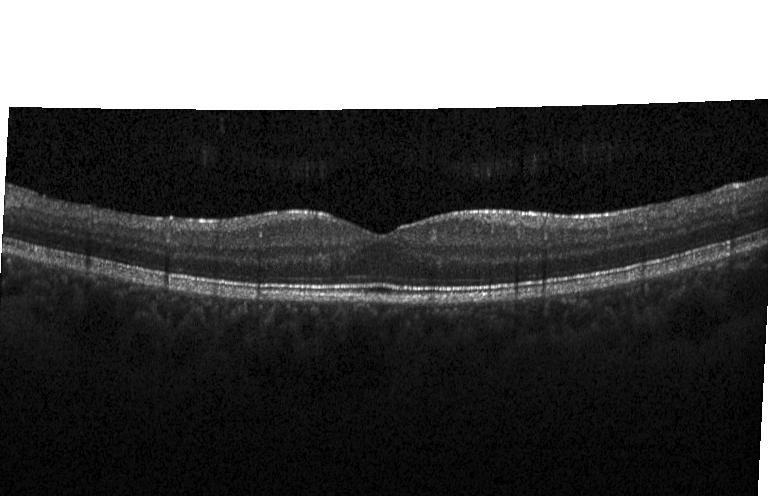

Instrument: Heidelberg Spectralis; through the macula; SD-OCT; OCT line scan. Diagnosis: no evidence of choroidal neovascularization, diabetic macular edema, or drusen.